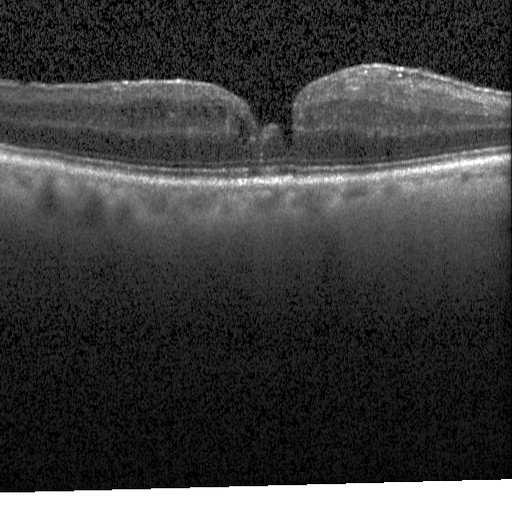
OCT B-scan.
Finding: diabetic macular edema (DME).